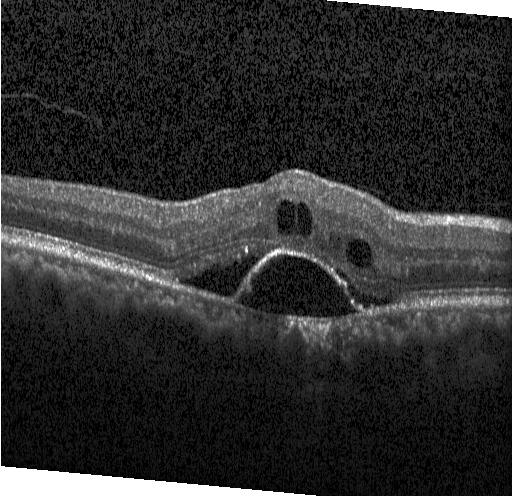 Assessment: choroidal neovascularization (CNV).